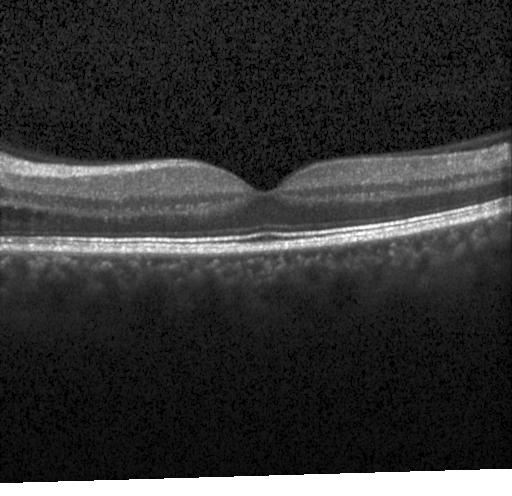

Spectral-domain OCT. Optical coherence tomography B-scan.
Diagnosis: no choroidal neovascularization, no diabetic macular edema, and no drusen.